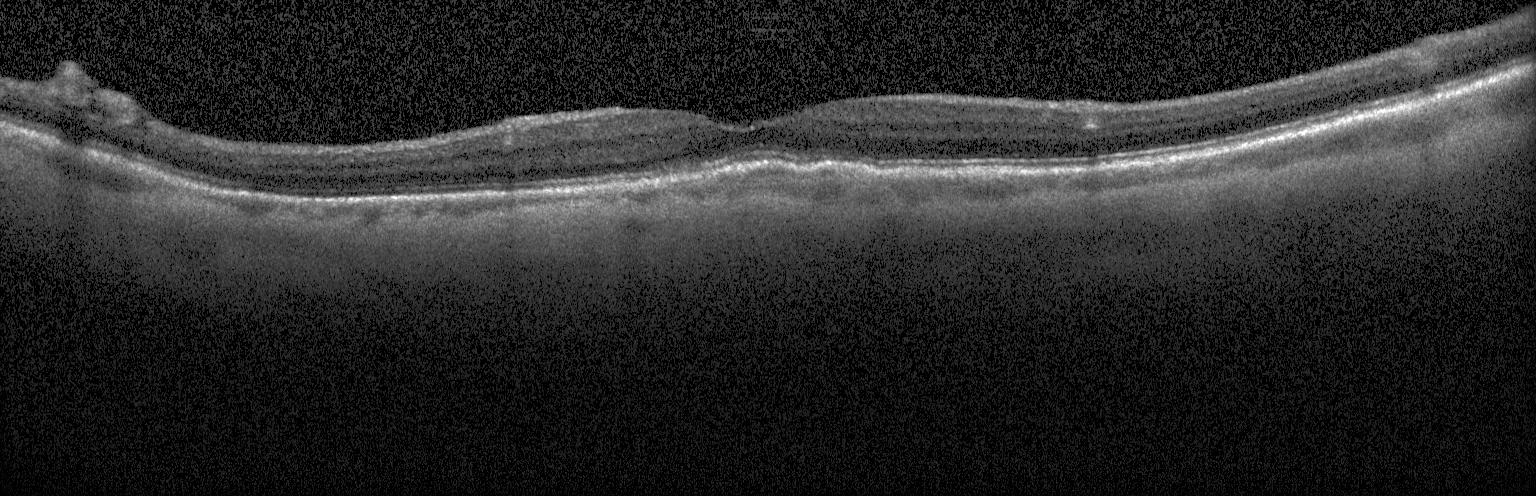

Horizontal scan through the fovea, retinal OCT B-scan
Assessment: choroidal neovascularization.